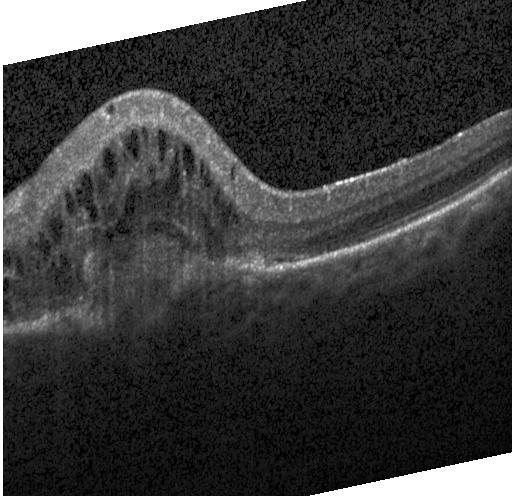 Through the macula · OCT line scan · spectral-domain optical coherence tomography.
OCT finding: CNV.